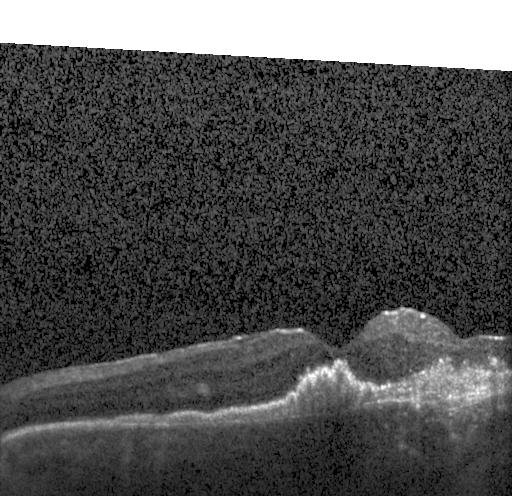
Macular OCT: choroidal neovascularization.